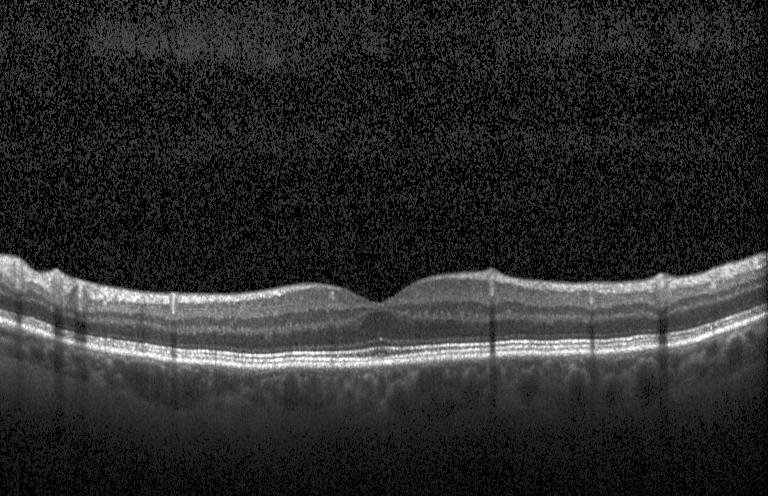
Optical coherence tomography B-scan
Dx: no CNV, no DME, and no drusen.